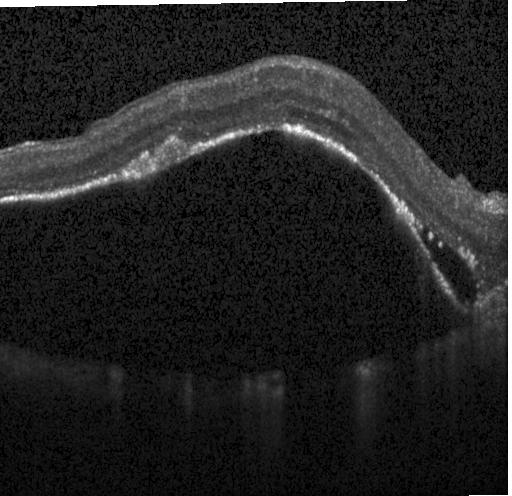 Choroidal neovascularization (CNV).